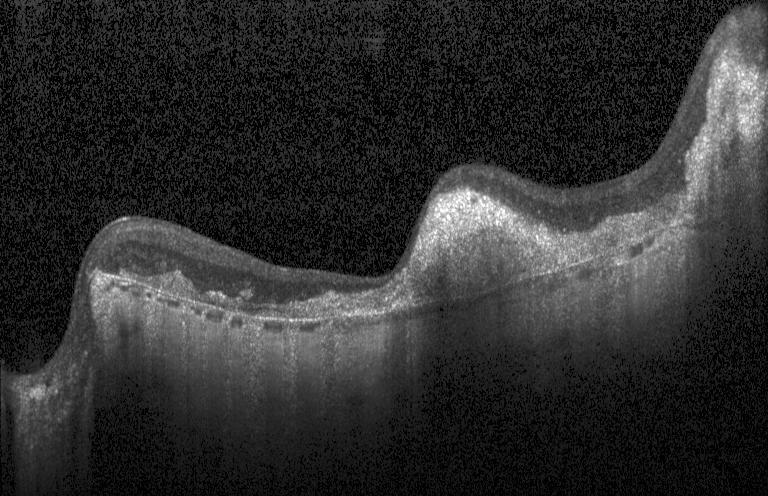 Acquired on a Heidelberg Spectralis; retinal OCT B-scan.
The scan shows a choroidal neovascular membrane.